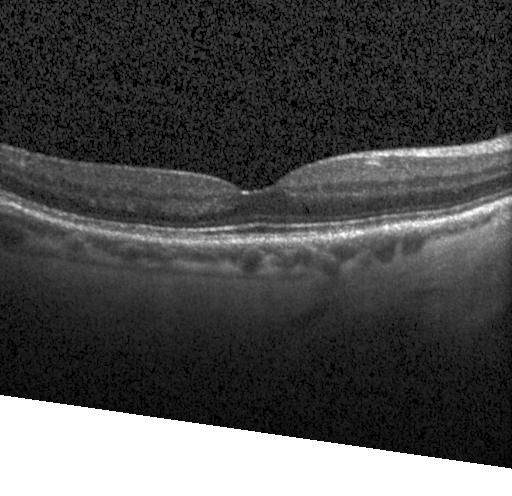 SD-OCT. Heidelberg Spectralis OCT system. Centered on the fovea. OCT B-scan.
Dx: no choroidal neovascularization, no diabetic macular edema, and no drusen.